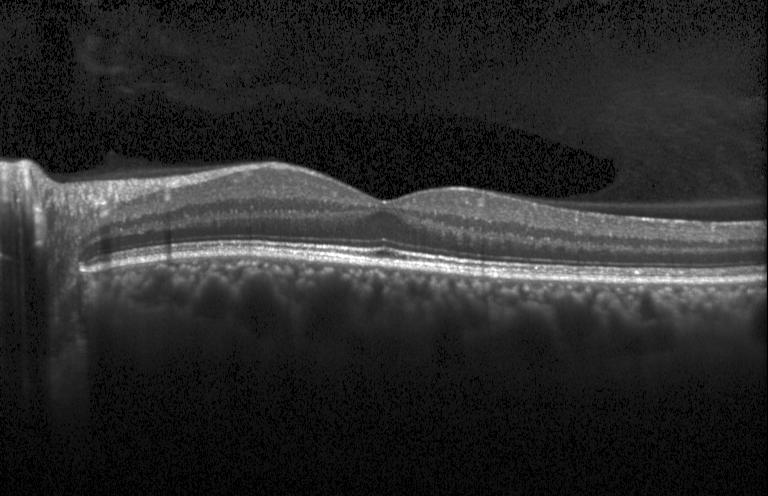
Through the macula · retinal OCT cross-section · Heidelberg Spectralis — Dx: neither CNV, DME, nor drusen.